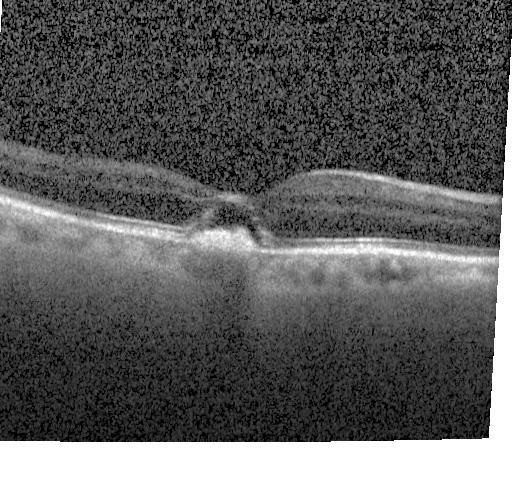 Instrument: Heidelberg Spectralis · optical coherence tomography B-scan · macular scan · SD-OCT
Finding: a choroidal neovascular membrane.